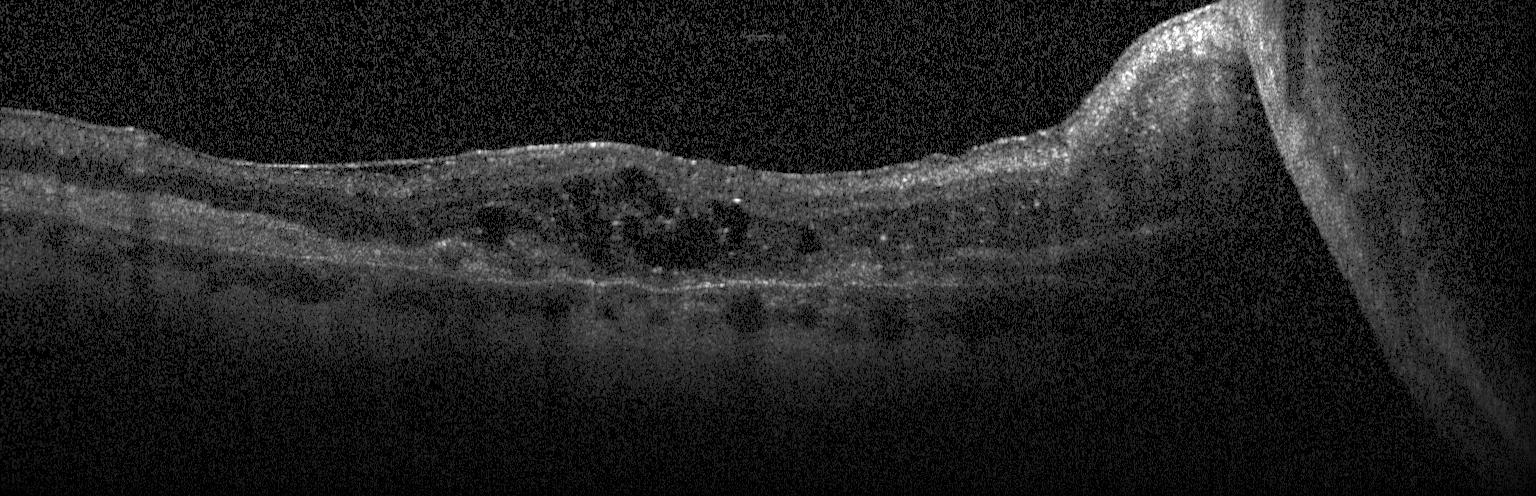
Macular OCT: CNV.